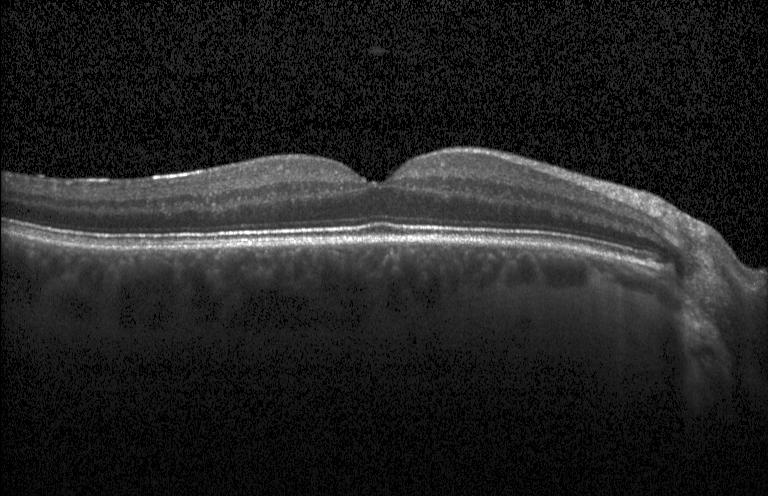 Retinal OCT cross-section. Heidelberg Spectralis OCT system. Centered on the fovea. Spectral-domain OCT.
This B-scan demonstrates no choroidal neovascularization, no diabetic macular edema, and no drusen.